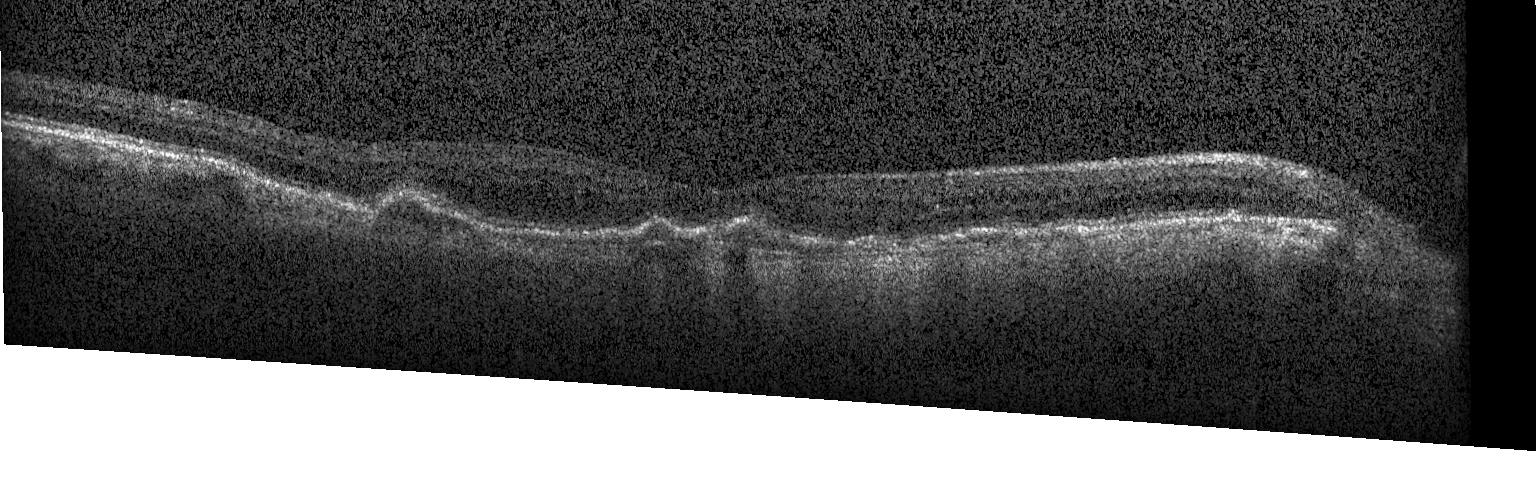 Impression: a choroidal neovascular membrane.